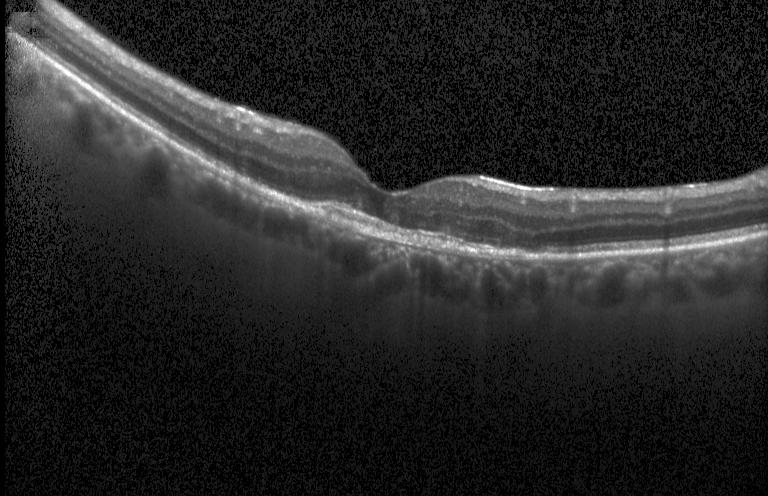

This B-scan demonstrates a choroidal neovascular membrane.